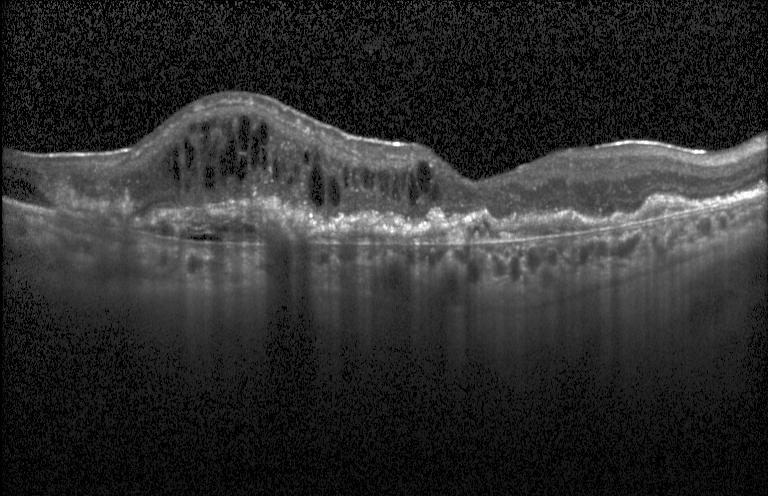
Macular OCT demonstrating CNV.